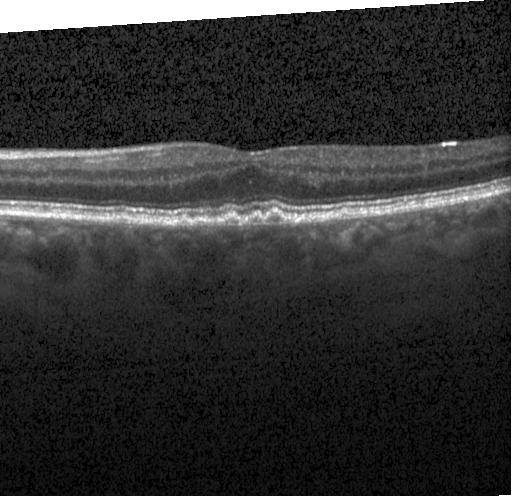

Finding: multiple drusen.